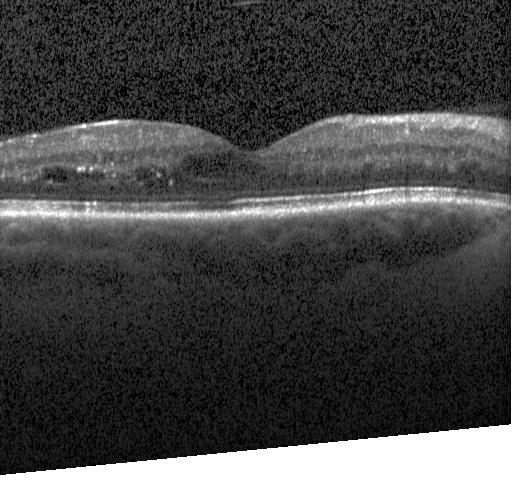 Optical coherence tomography B-scan.
Diagnosis: diabetic macular edema (DME).